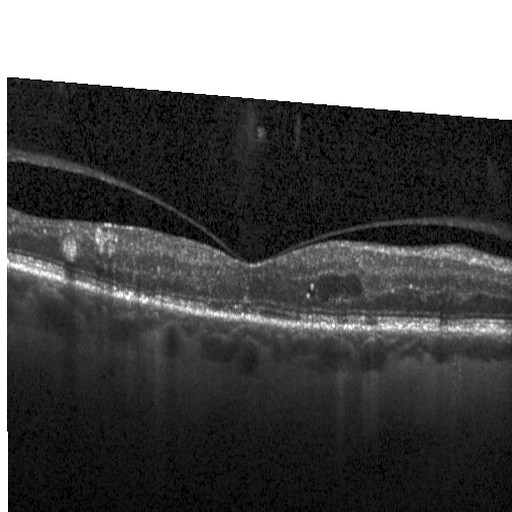 Heidelberg Spectralis OCT system. Optical coherence tomography B-scan. Horizontal scan through the fovea — Impression: diabetic macular edema (DME).